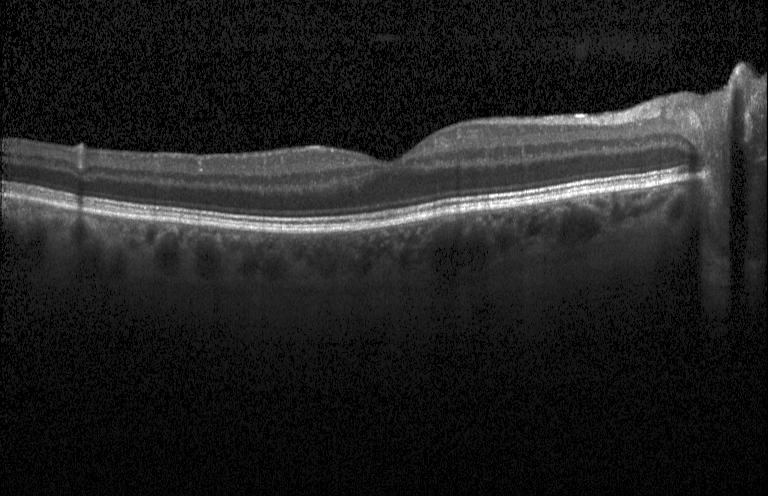

Finding: no evidence of choroidal neovascularization, diabetic macular edema, or drusen.